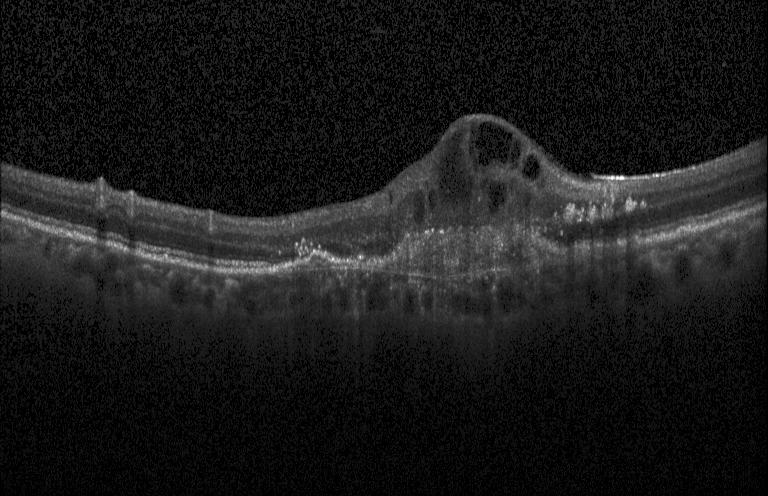 Optical coherence tomography scan, SD-OCT — OCT finding: choroidal neovascularization.